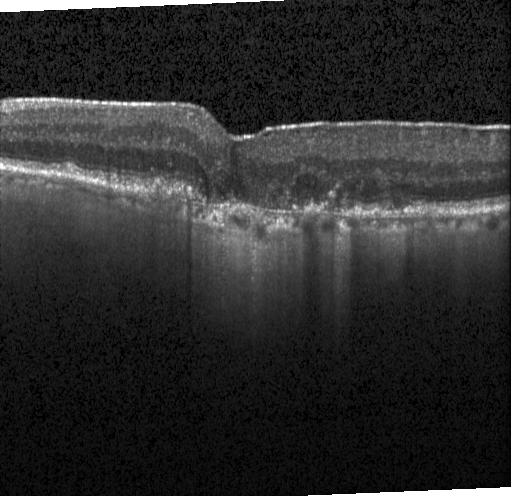
OCT scan showing choroidal neovascularization.